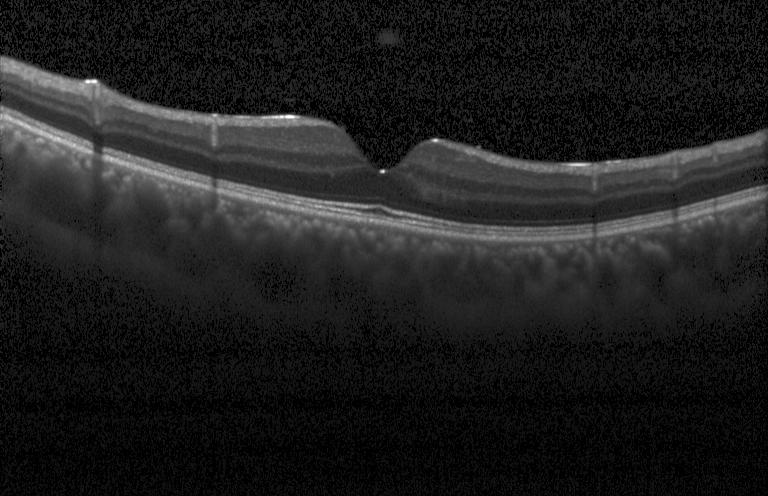

Spectral-domain optical coherence tomography; macular scan; OCT line scan; Heidelberg Spectralis OCT system
OCT finding: no evidence of choroidal neovascularization, diabetic macular edema, or drusen.